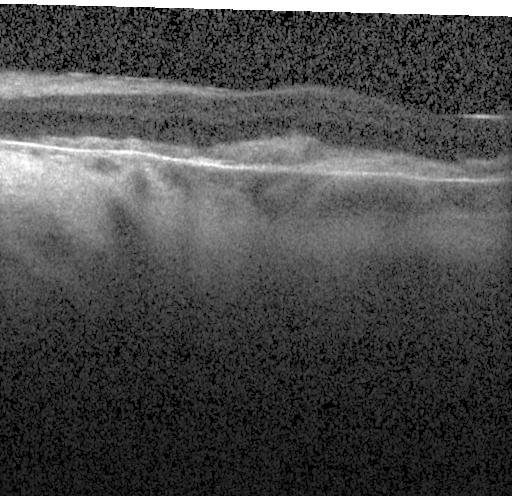
The scan shows choroidal neovascularization.